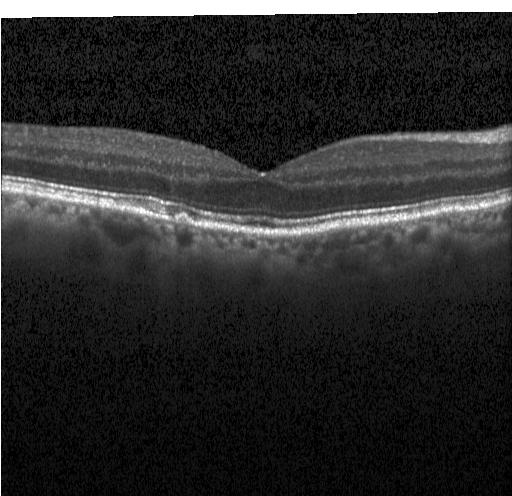

OCT scan showing sub-RPE drusenoid deposits.